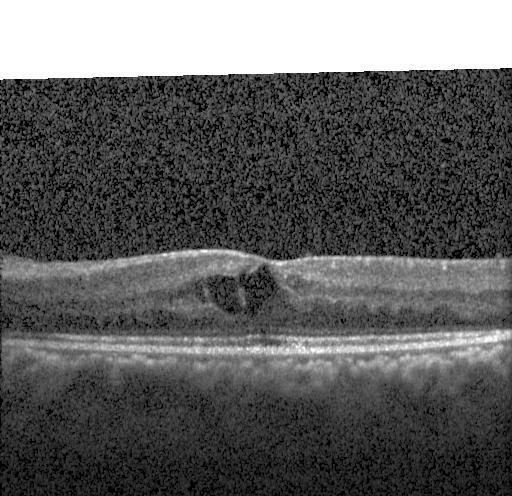 Dx: diabetic macular edema.